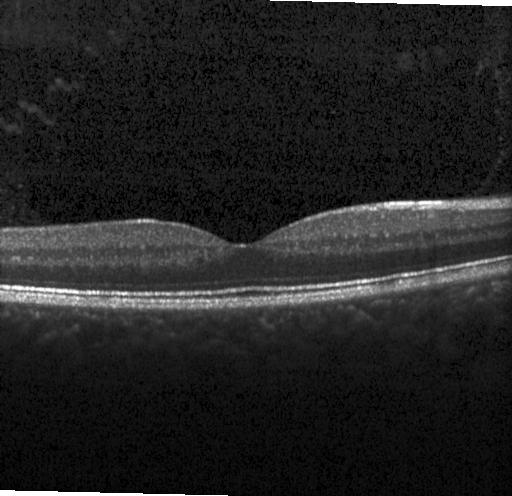 Retinal OCT B-scan · spectral-domain OCT · centered on the fovea · acquired on a Heidelberg Spectralis.
Impression: no choroidal neovascularization, diabetic macular edema, or drusen.